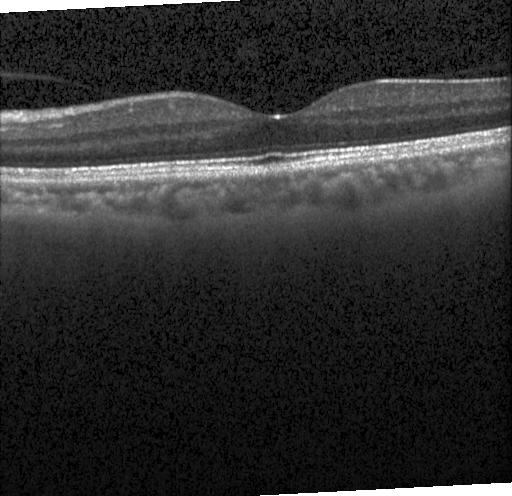

Retinal OCT cross-section, macular scan
Dx: no choroidal neovascularization, diabetic macular edema, or drusen.